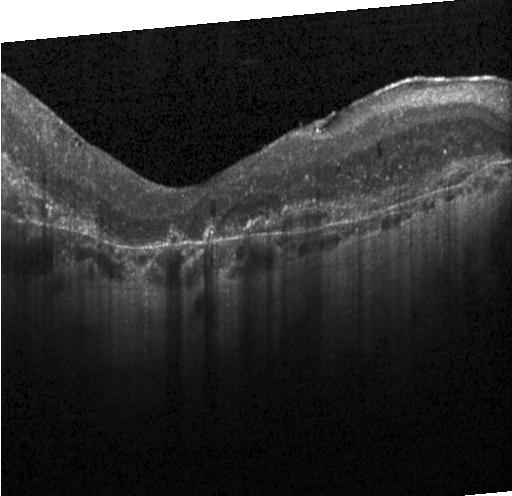

Retinal OCT B-scan · spectral-domain OCT · instrument: Heidelberg Spectralis. Finding: choroidal neovascularization.